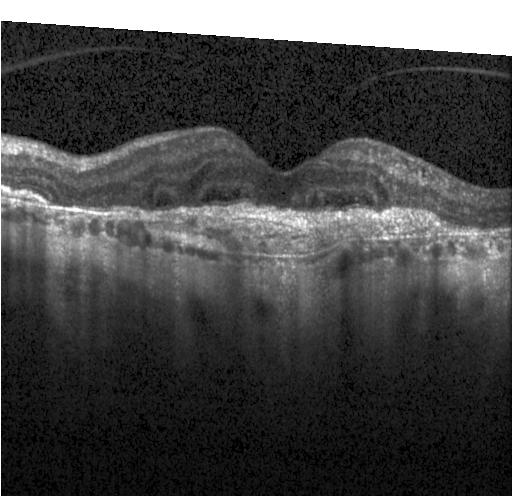

SD-OCT, retinal OCT cross-section. Diagnosis: a choroidal neovascular membrane.